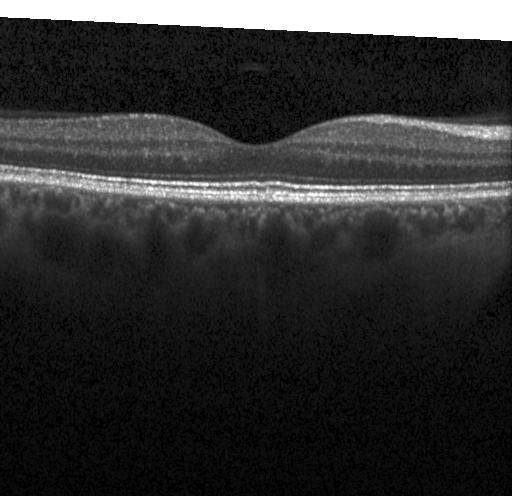 Optical coherence tomography B-scan.
Impression: no choroidal neovascularization, diabetic macular edema, or drusen.